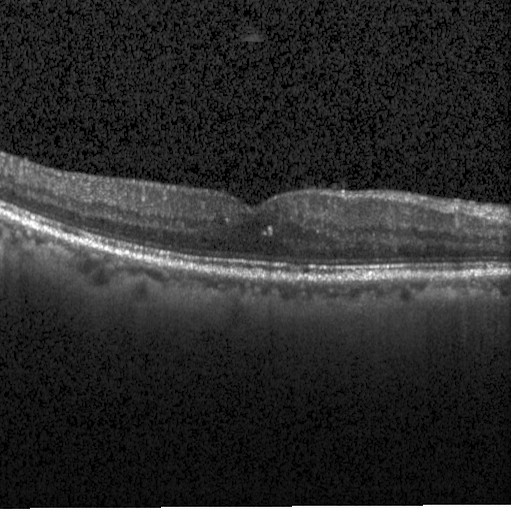

The scan shows DME.